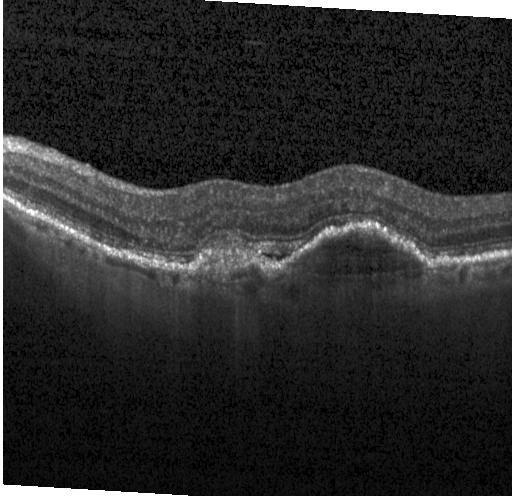 Retinal OCT cross-section; fovea-centered; spectral-domain OCT; acquired on a Heidelberg Spectralis.
A choroidal neovascular membrane.